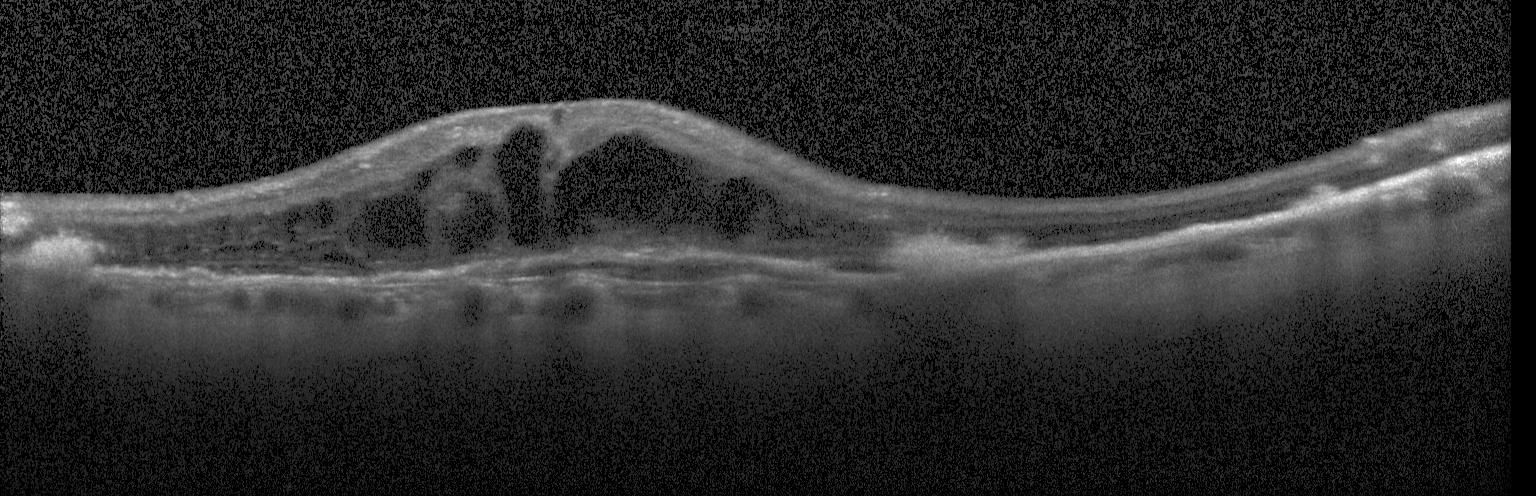 OCT line scan; macular scan; Heidelberg Spectralis — Dx: a choroidal neovascular membrane.